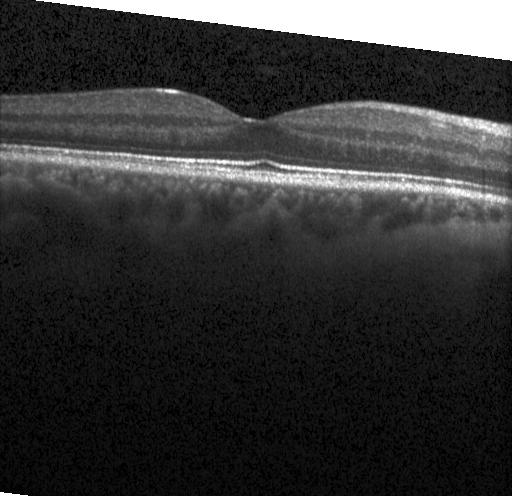 Finding: no CNV, DME, or drusen.